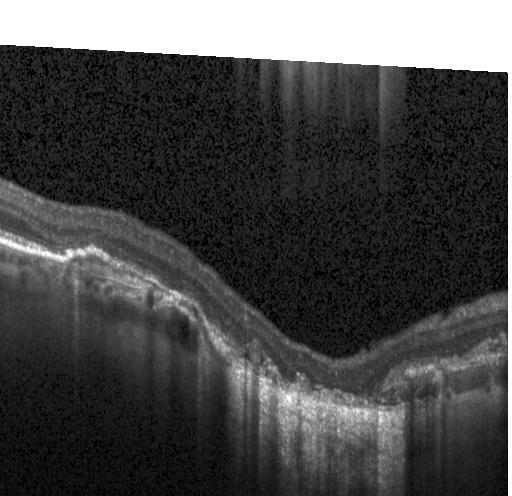

Diagnosis: a choroidal neovascular membrane.